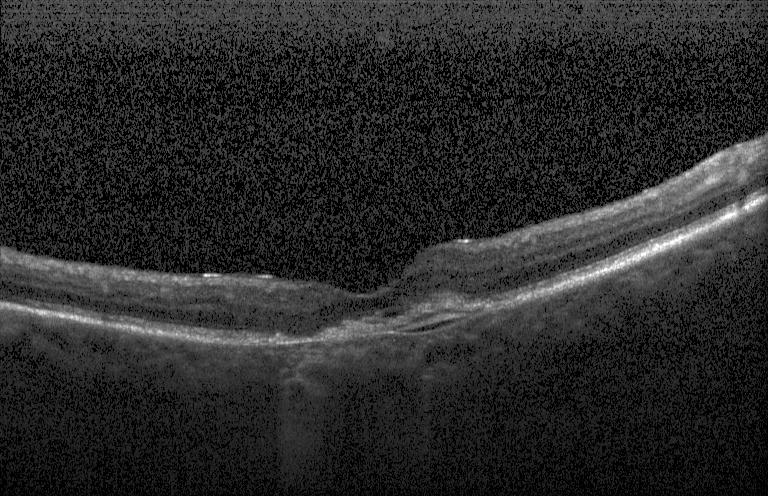

Dx: a choroidal neovascular membrane.